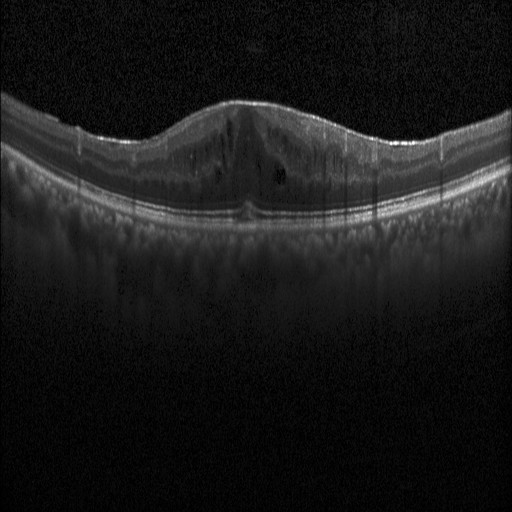 OCT B-scan · Heidelberg Spectralis OCT system · macular scan · spectral-domain OCT. Impression: diabetic macular edema (DME).